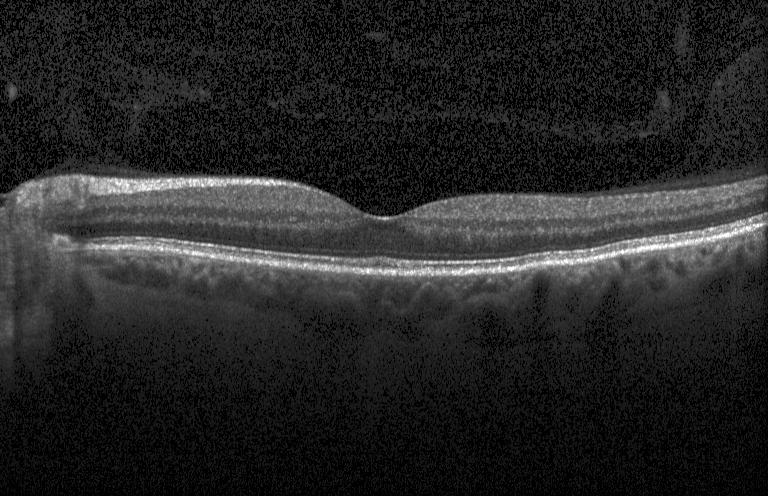

Retinal OCT B-scan · horizontal scan through the fovea · instrument: Heidelberg Spectralis
The scan shows neither choroidal neovascularization, diabetic macular edema, nor drusen.